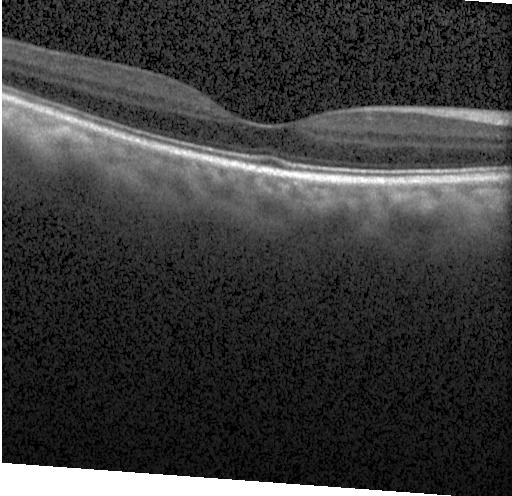 Retinal OCT cross-section.
No evidence of choroidal neovascularization, diabetic macular edema, or drusen.